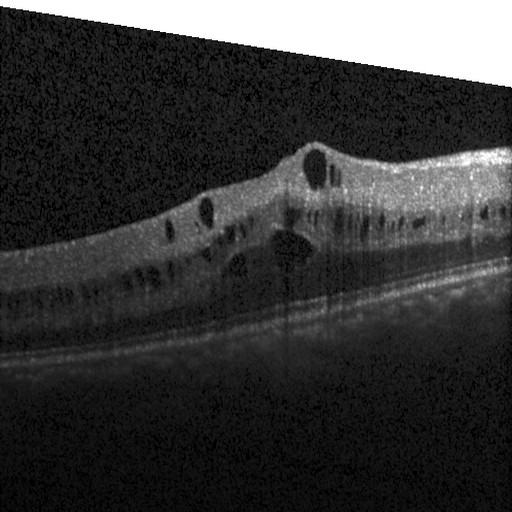

Centered on the fovea, OCT B-scan, spectral-domain OCT.
Diagnosis: diabetic macular edema (DME).